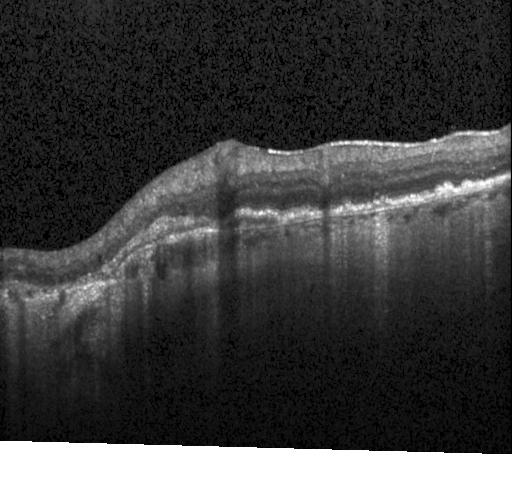
Retinal OCT cross-section · Heidelberg Spectralis.
Diagnosis: choroidal neovascularization (CNV).